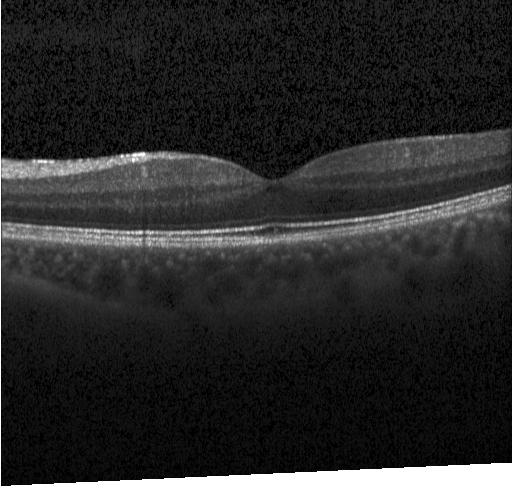
The scan shows no choroidal neovascularization, diabetic macular edema, or drusen.